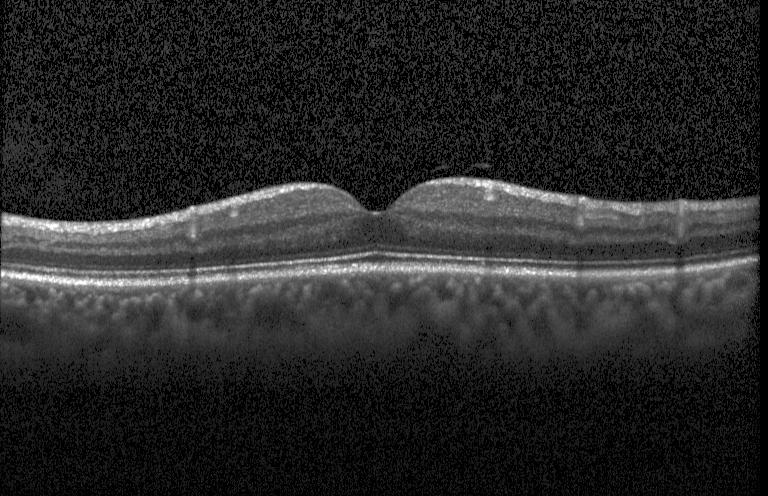
SD-OCT, OCT B-scan — Impression: no evidence of choroidal neovascularization, diabetic macular edema, or drusen.